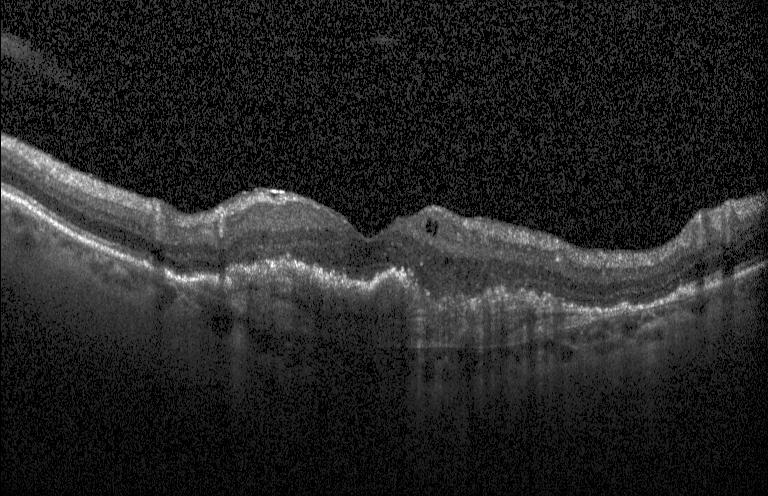
A choroidal neovascular membrane.